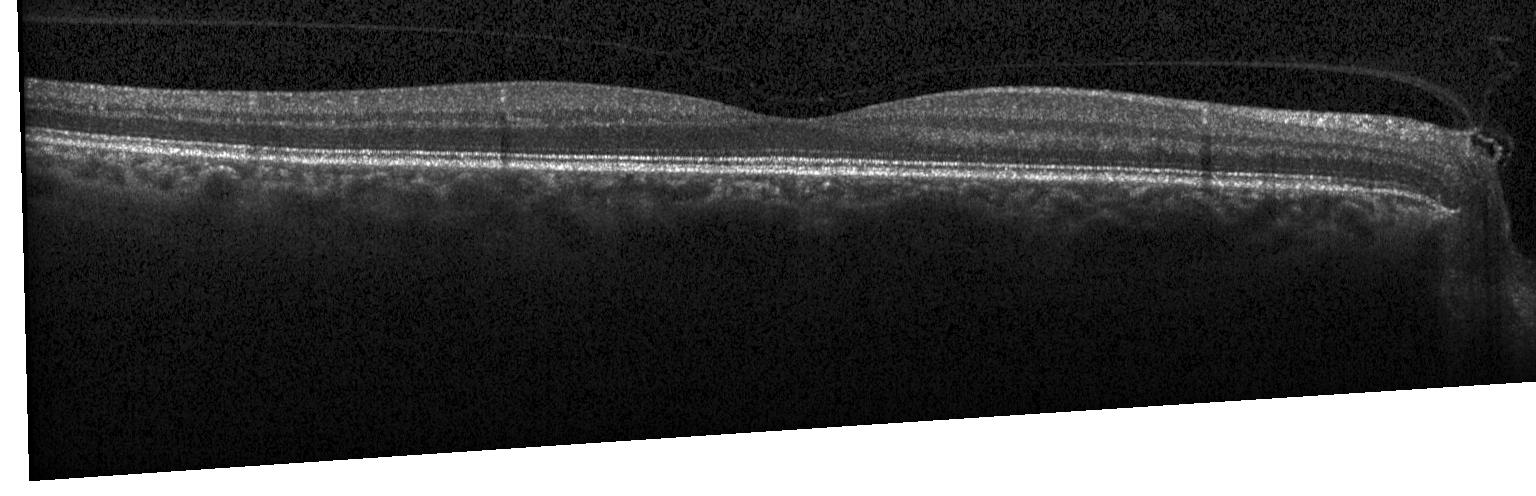

Diagnosis: no choroidal neovascularization, no diabetic macular edema, and no drusen.